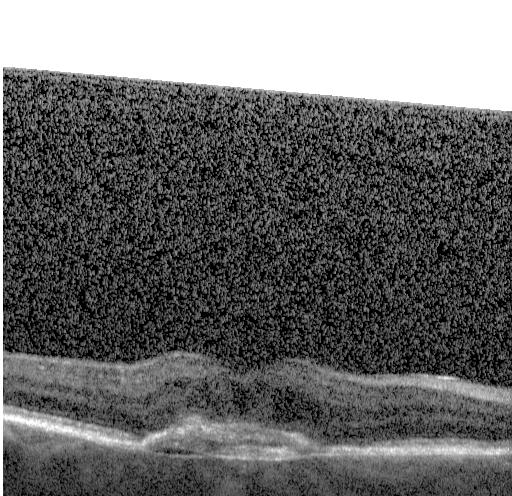

OCT finding: a choroidal neovascular membrane.